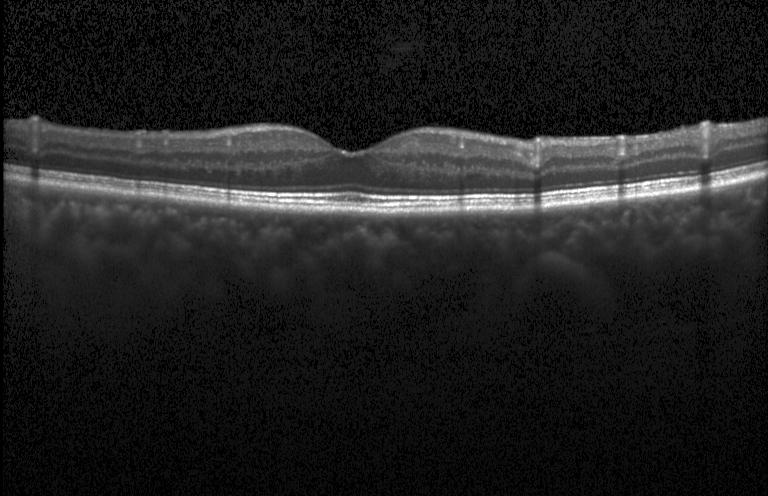
Acquired on a Heidelberg Spectralis. Retinal OCT B-scan. Macular scan. SD-OCT. Impression: no choroidal neovascularization, diabetic macular edema, or drusen.